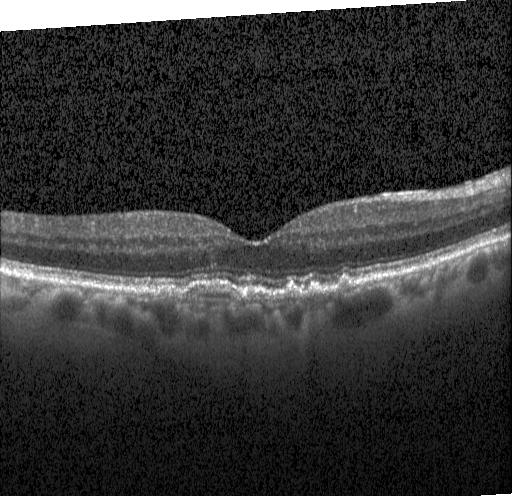

Retinal OCT cross-section, instrument: Heidelberg Spectralis. Impression: sub-RPE drusenoid deposits.